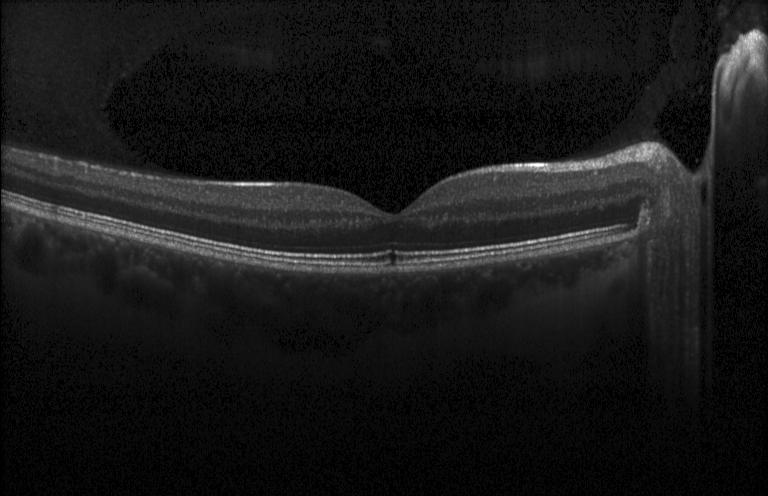
Horizontal scan through the fovea. Heidelberg Spectralis OCT system. Retinal OCT B-scan. Spectral-domain optical coherence tomography
Impression: no CNV, no DME, and no drusen.